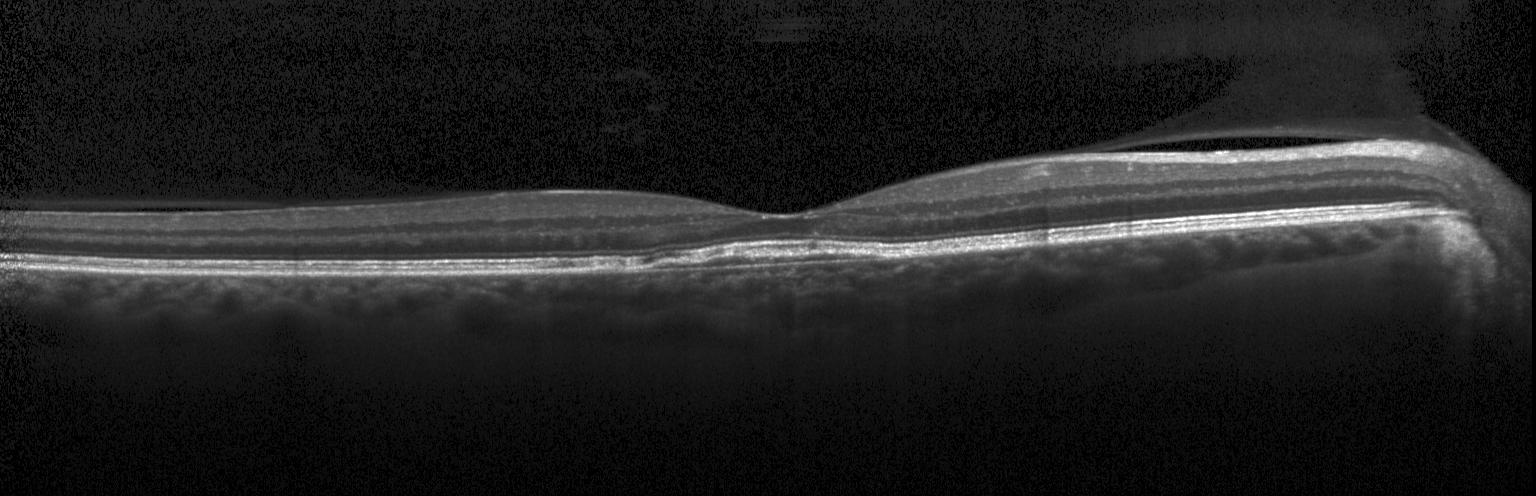

Impression: choroidal neovascularization.